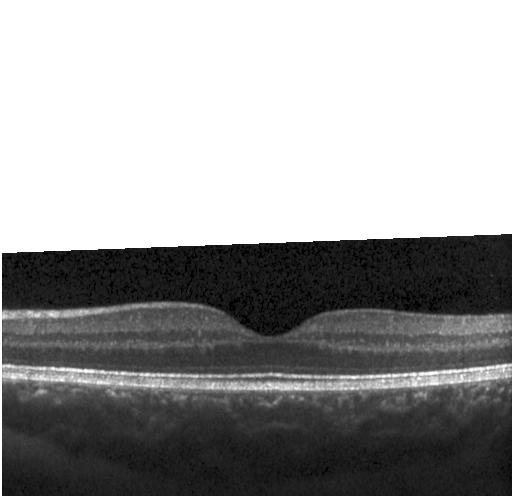
OCT scan showing no choroidal neovascularization, no diabetic macular edema, and no drusen.